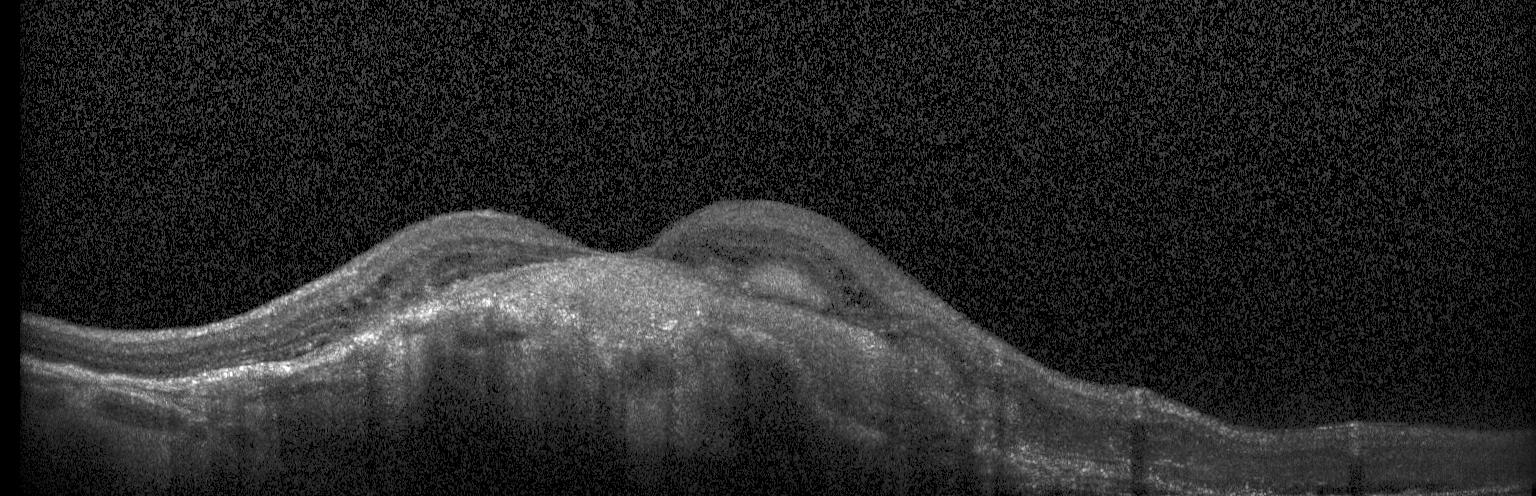
Heidelberg Spectralis OCT system · through the macula · optical coherence tomography B-scan · SD-OCT
Finding: choroidal neovascularization.